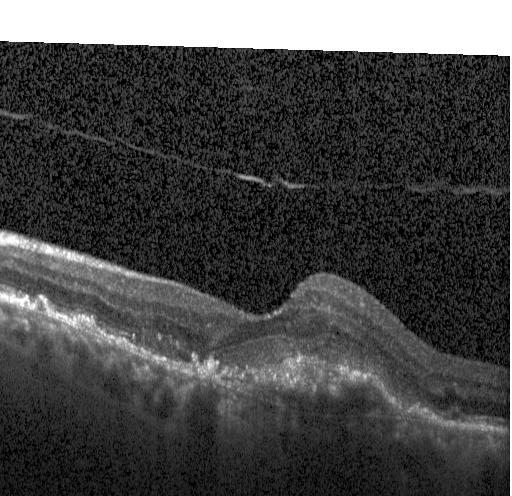
Heidelberg Spectralis OCT system, spectral-domain optical coherence tomography, retinal OCT cross-section.
A choroidal neovascular membrane.